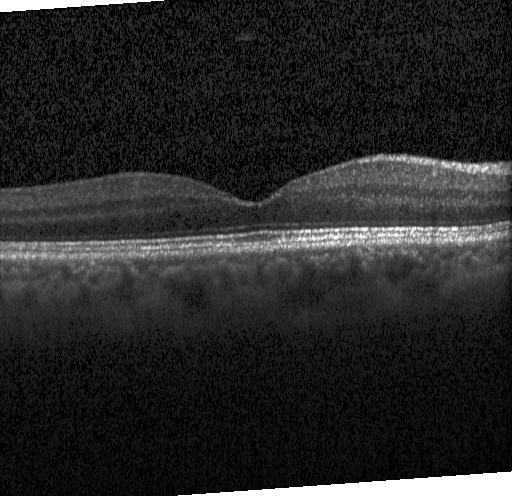

Instrument: Heidelberg Spectralis, SD-OCT, OCT B-scan, fovea-centered — Impression: no evidence of CNV, DME, or drusen.